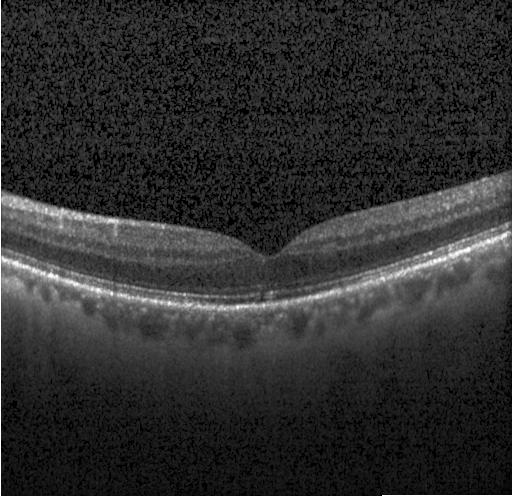 Heidelberg Spectralis OCT system, OCT B-scan, macular scan — Finding: no evidence of choroidal neovascularization, diabetic macular edema, or drusen.